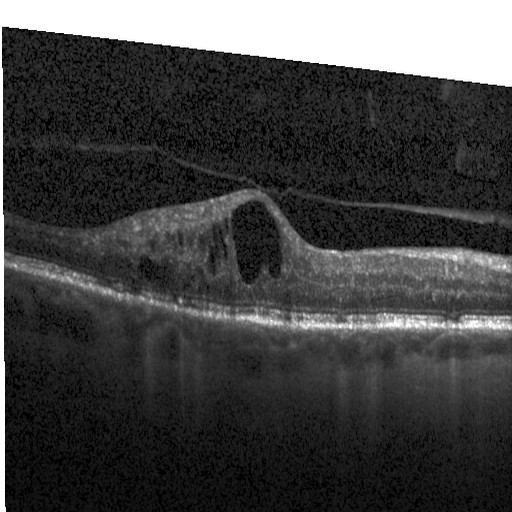

OCT line scan. Instrument: Heidelberg Spectralis
Diagnosis: diabetic macular edema (DME).